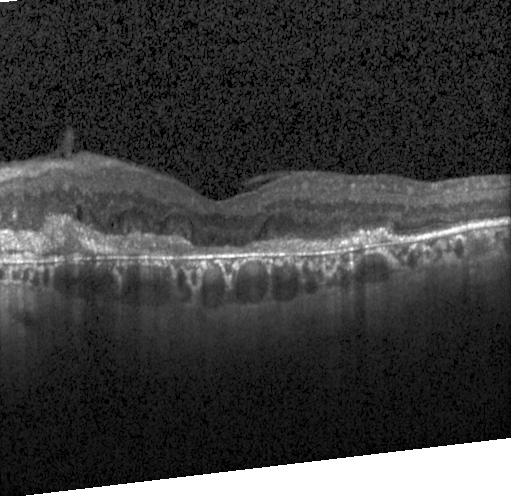

OCT B-scan.
Finding: choroidal neovascularization.